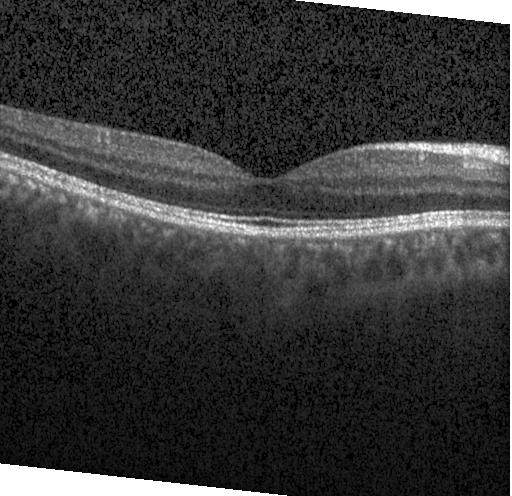 Assessment: no CNV, DME, or drusen.